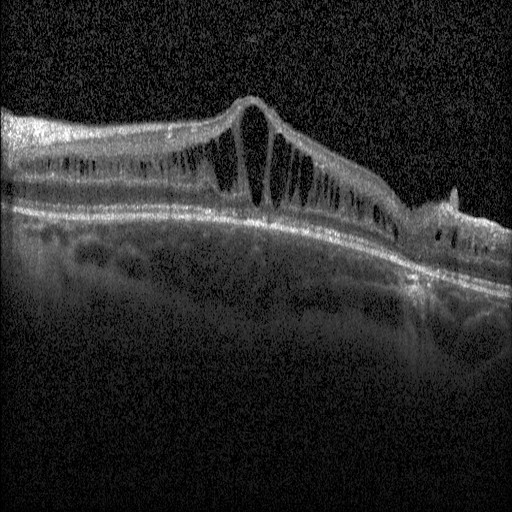
Finding: diabetic macular edema.